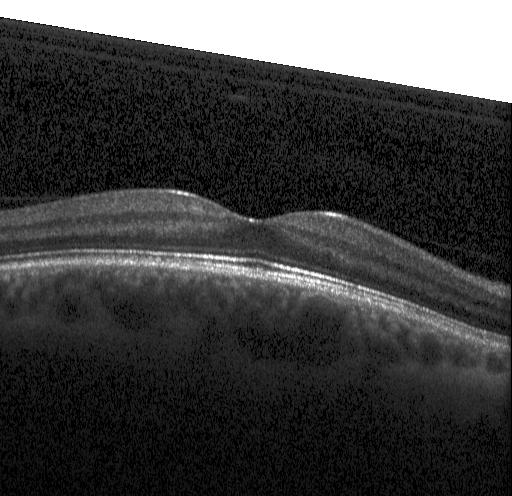
Impression: no choroidal neovascularization, diabetic macular edema, or drusen.